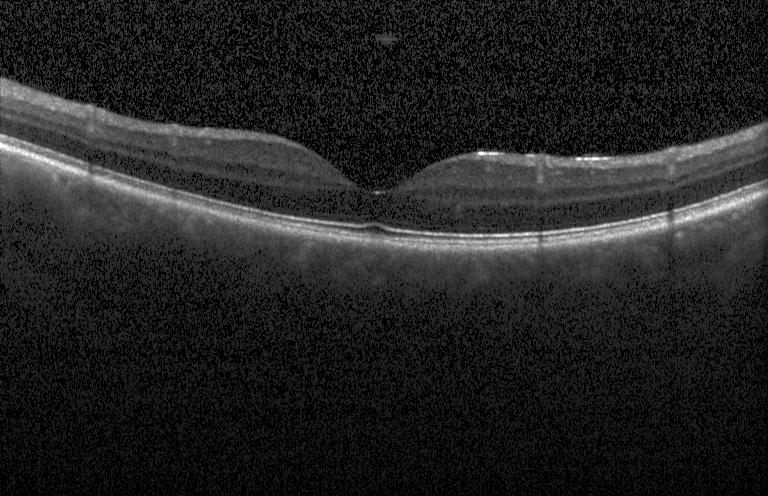 No CNV, DME, or drusen.